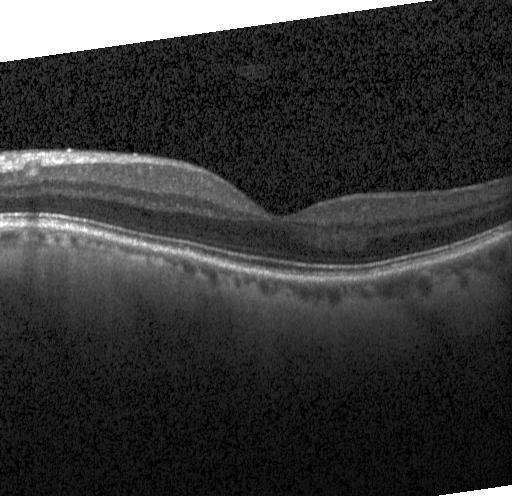 Instrument: Heidelberg Spectralis, OCT line scan, spectral-domain optical coherence tomography, macular scan.
Dx: neither choroidal neovascularization, diabetic macular edema, nor drusen.